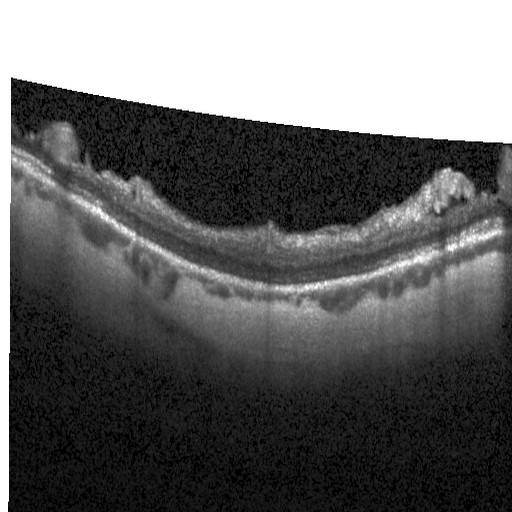

OCT B-scan — Impression: diabetic macular edema (DME).